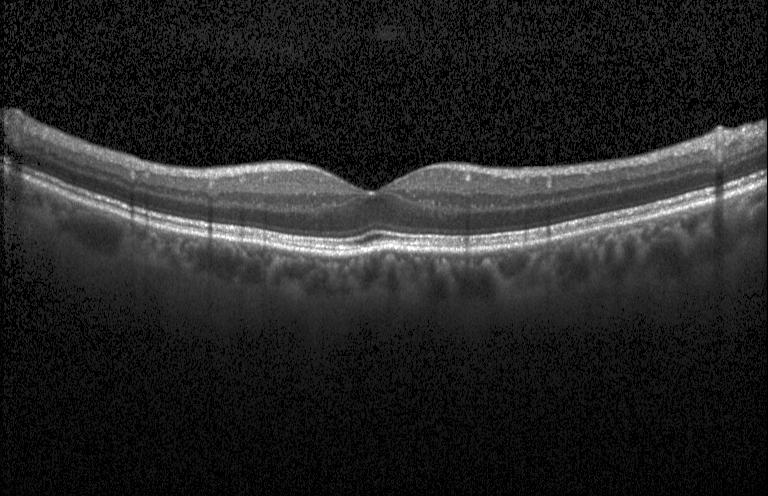
Diagnosis: no evidence of CNV, DME, or drusen.